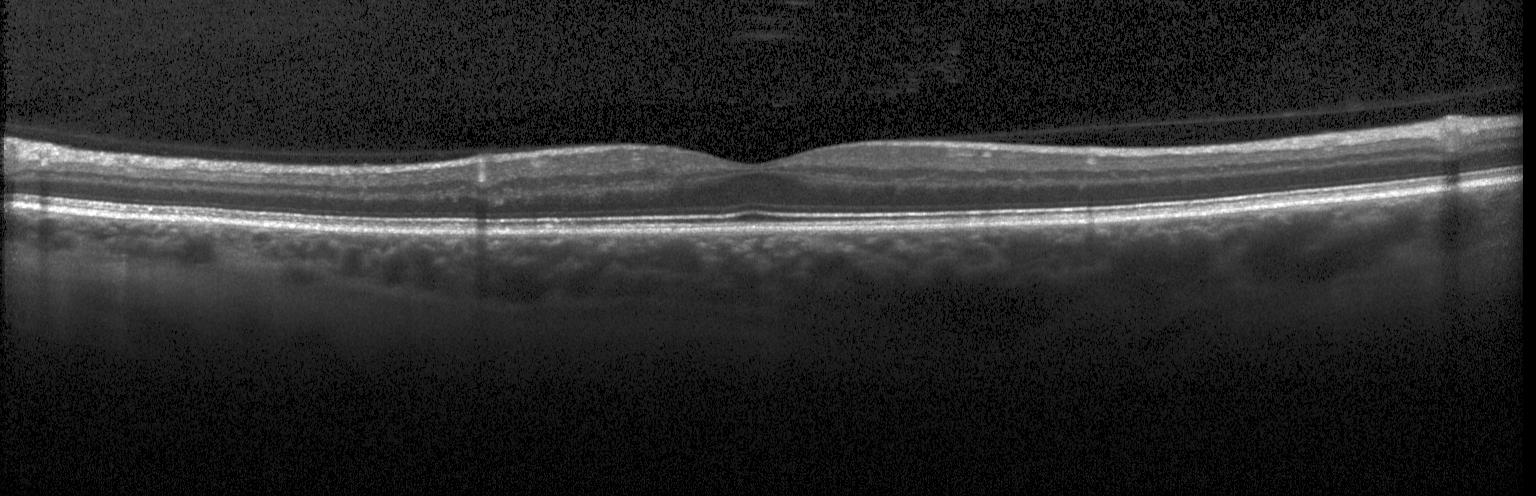 The scan shows neither choroidal neovascularization, diabetic macular edema, nor drusen.